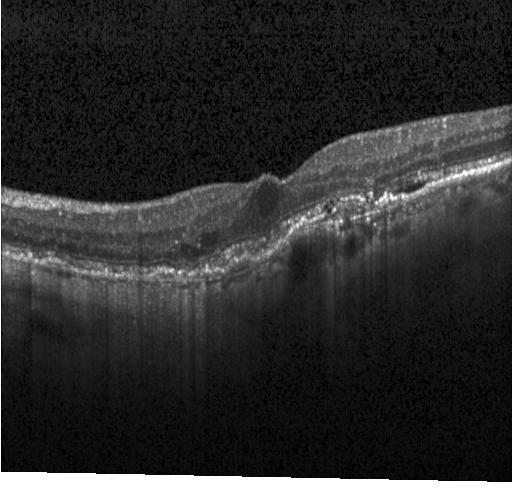
Macular scan; optical coherence tomography B-scan; acquired on a Heidelberg Spectralis
Diagnosis: choroidal neovascularization.